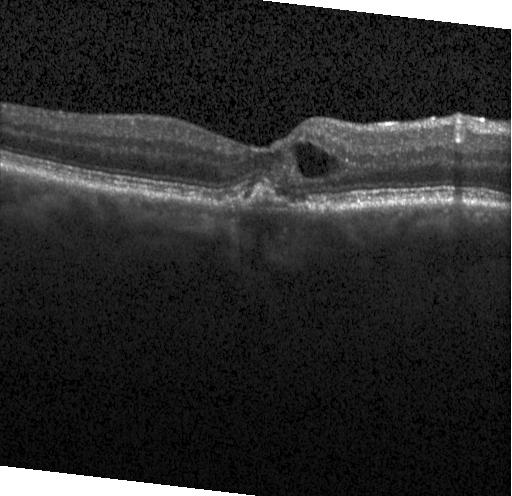

Optical coherence tomography scan — Finding: a choroidal neovascular membrane.